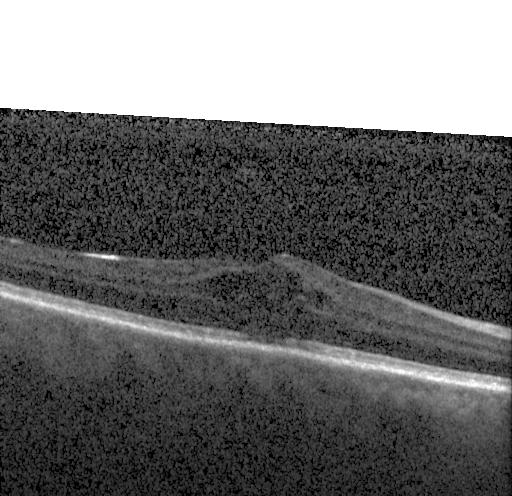
Instrument: Heidelberg Spectralis · horizontal scan through the fovea · retinal OCT B-scan · spectral-domain optical coherence tomography — Finding: diabetic macular edema (DME).